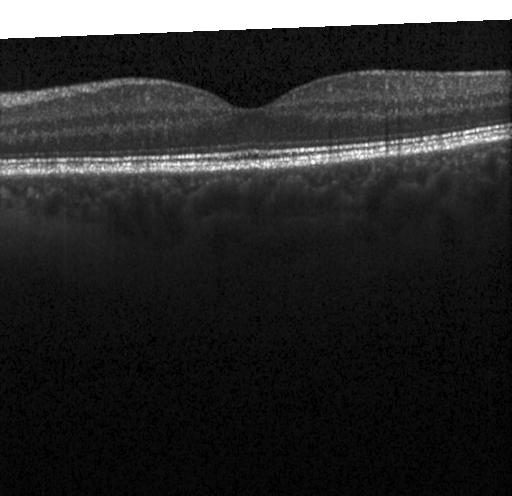 Retinal OCT cross-section — OCT finding: neither choroidal neovascularization, diabetic macular edema, nor drusen.